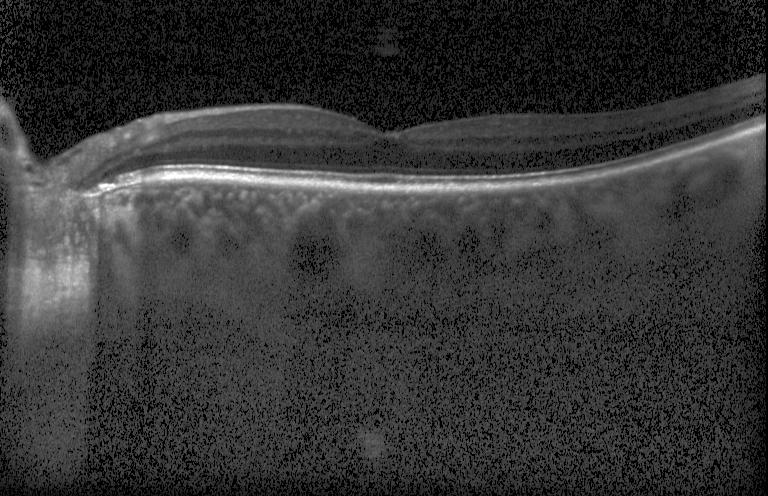 No CNV, no DME, and no drusen.